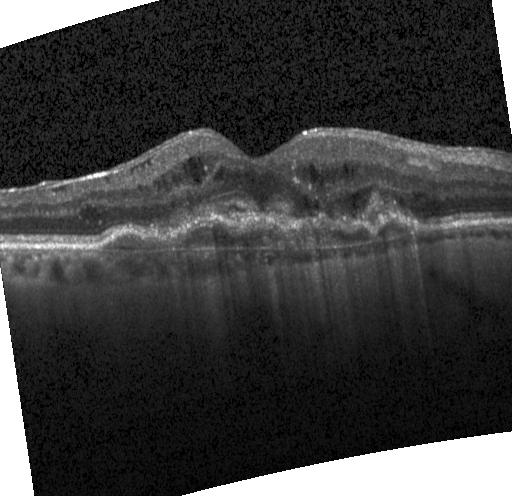 Retinal OCT cross-section.
Dx: a choroidal neovascular membrane.